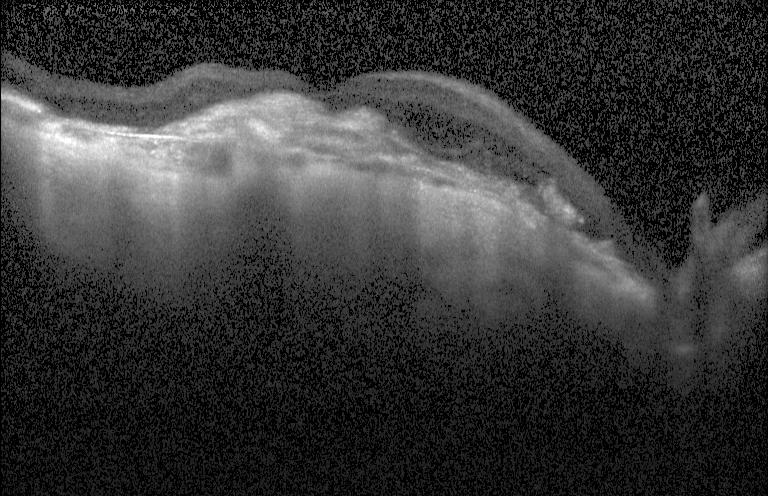

Acquired on a Heidelberg Spectralis, optical coherence tomography scan. Assessment: choroidal neovascularization.